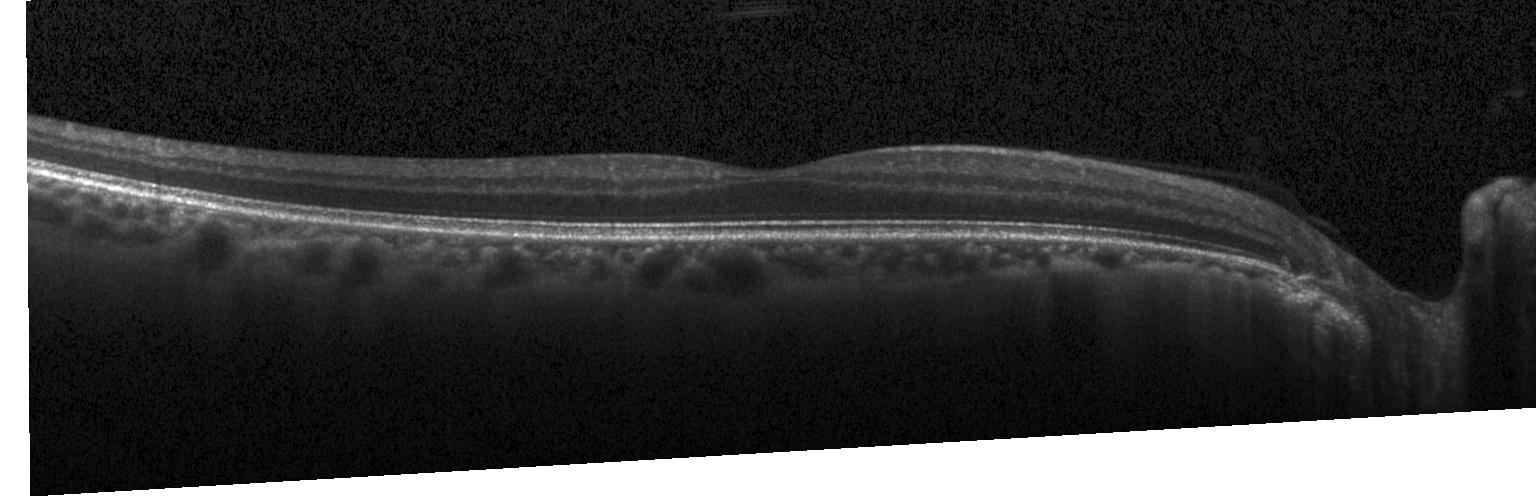 OCT B-scan. Acquired on a Heidelberg Spectralis. No evidence of CNV, DME, or drusen.